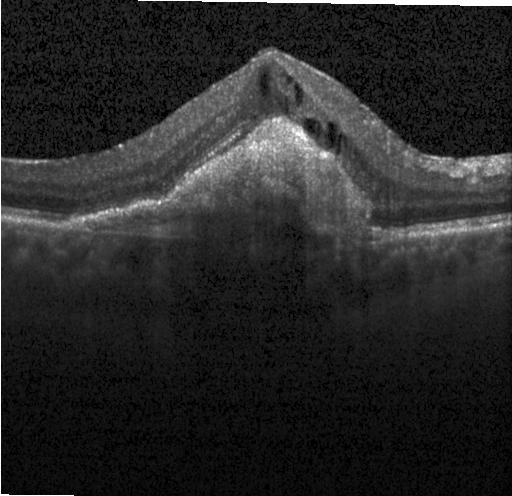
SD-OCT; retinal OCT B-scan; through the macula; acquired on a Heidelberg Spectralis.
This B-scan demonstrates choroidal neovascularization (CNV).